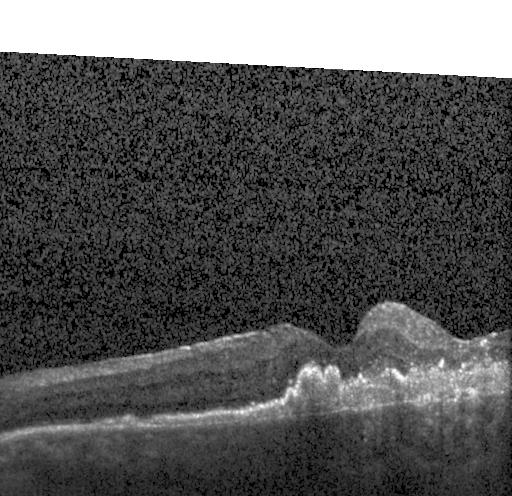
Impression: choroidal neovascularization.